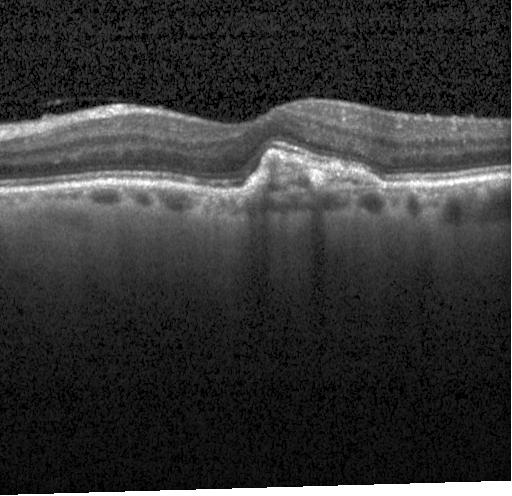

Heidelberg Spectralis, macular scan, OCT line scan.
Impression: CNV.